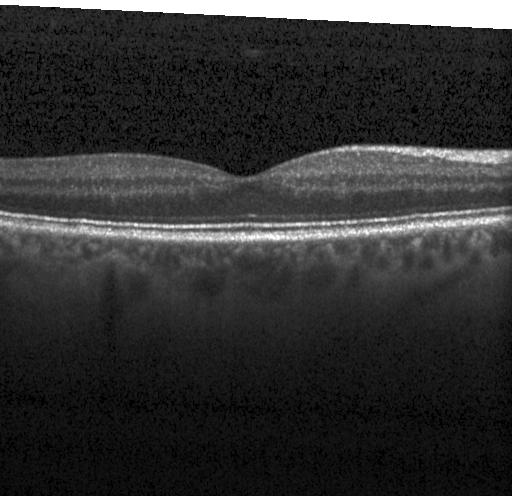 OCT B-scan · spectral-domain optical coherence tomography · centered on the fovea.
Macular OCT: no evidence of choroidal neovascularization, diabetic macular edema, or drusen.